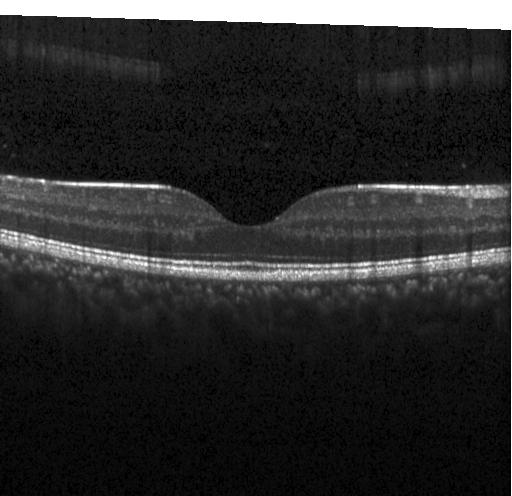 Macular scan · spectral-domain OCT · Heidelberg Spectralis OCT system · OCT B-scan
Finding: no choroidal neovascularization, diabetic macular edema, or drusen.